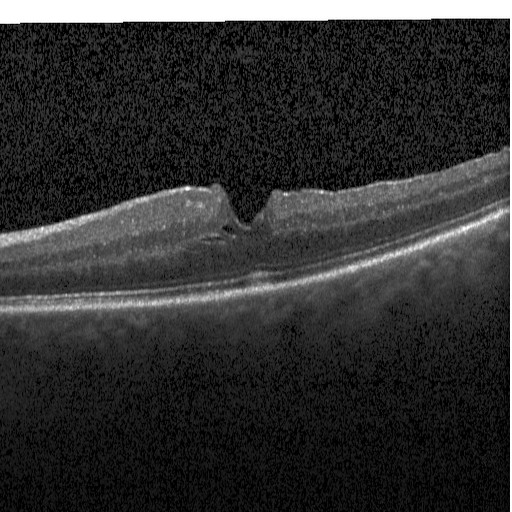 OCT B-scan showing diabetic macular edema (DME).